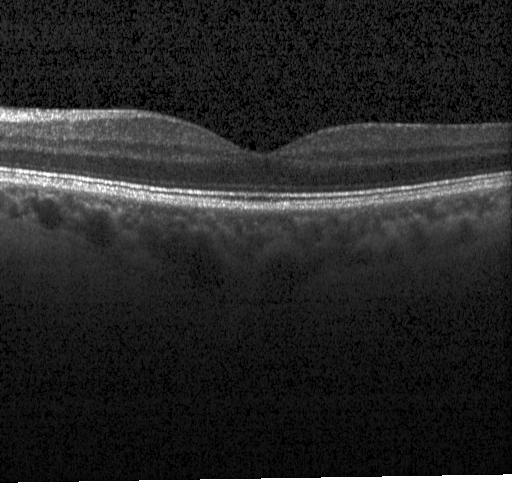
Retinal OCT cross-section showing no choroidal neovascularization, diabetic macular edema, or drusen.